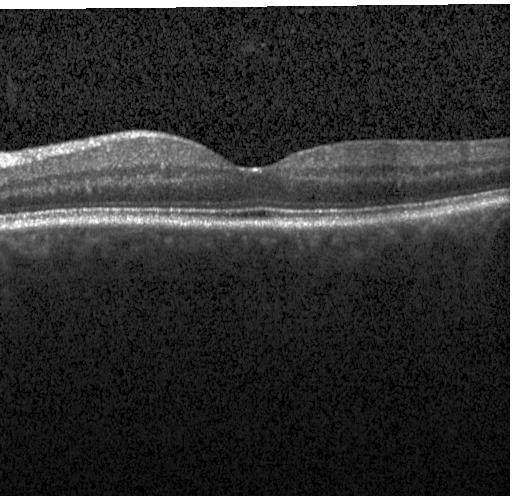

Macular scan, retinal OCT cross-section
No choroidal neovascularization, diabetic macular edema, or drusen.